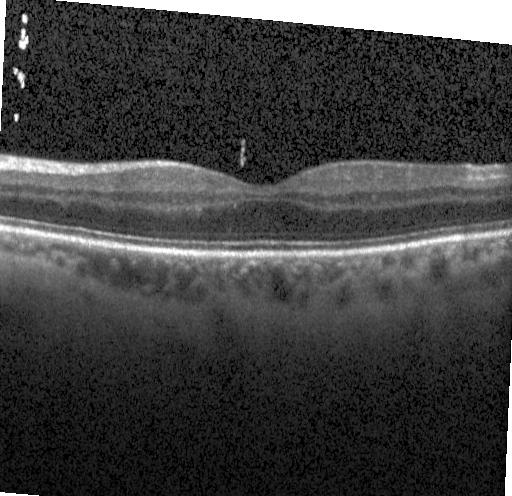

Optical coherence tomography B-scan, fovea-centered
No choroidal neovascularization, no diabetic macular edema, and no drusen.